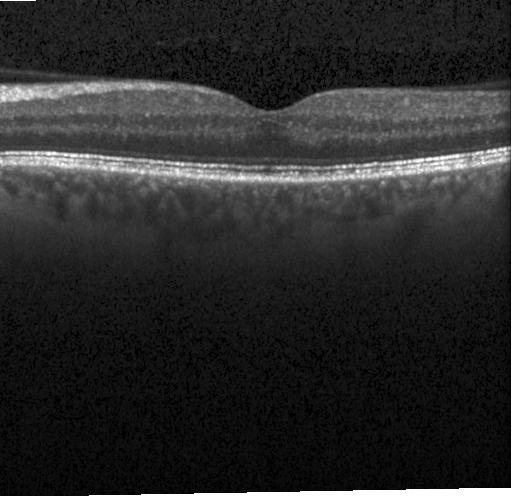

Through the macula. OCT line scan. Heidelberg Spectralis
No choroidal neovascularization, no diabetic macular edema, and no drusen.